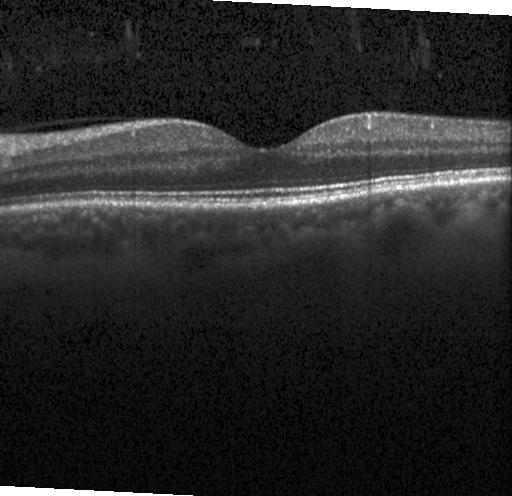
Optical coherence tomography B-scan. Heidelberg Spectralis.
Impression: no choroidal neovascularization, diabetic macular edema, or drusen.